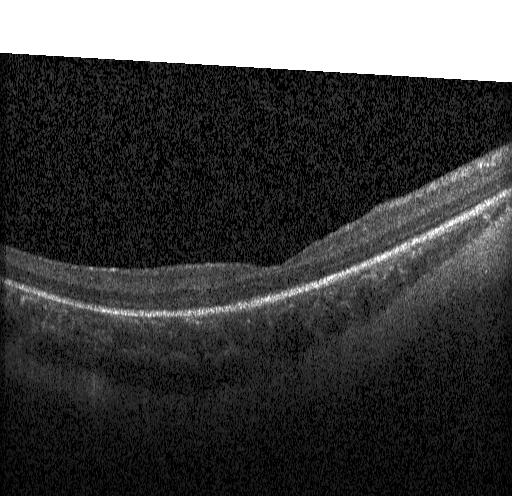 Instrument: Heidelberg Spectralis · through the macula · spectral-domain optical coherence tomography · optical coherence tomography scan — Diagnosis: no CNV, no DME, and no drusen.